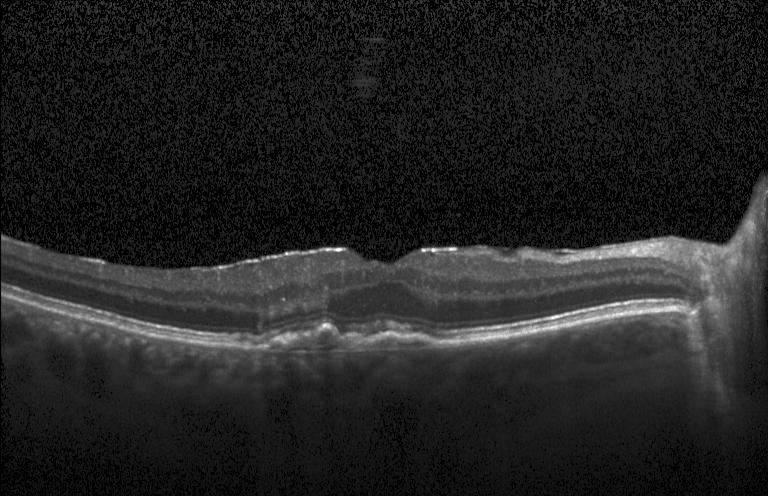
Optical coherence tomography B-scan
Diagnosis: a choroidal neovascular membrane.